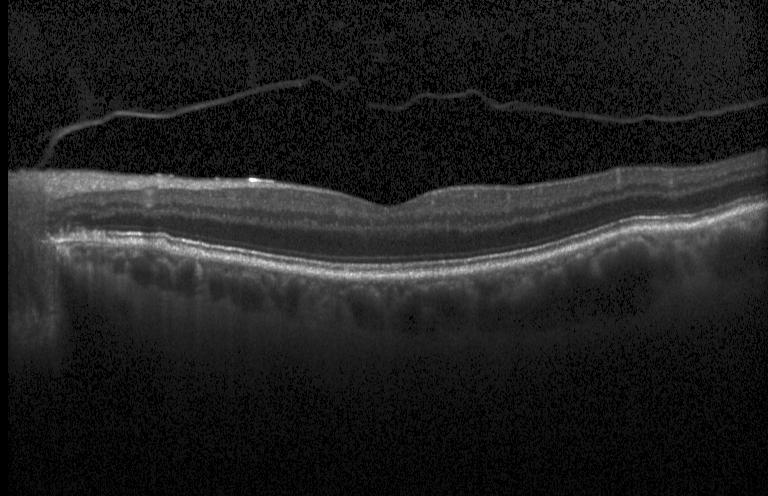 Heidelberg Spectralis OCT system, horizontal scan through the fovea, SD-OCT, retinal OCT cross-section — Macular OCT: neither CNV, DME, nor drusen.